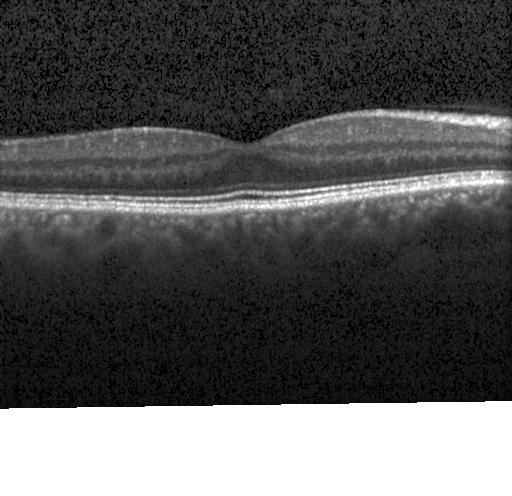 The scan shows no evidence of choroidal neovascularization, diabetic macular edema, or drusen.